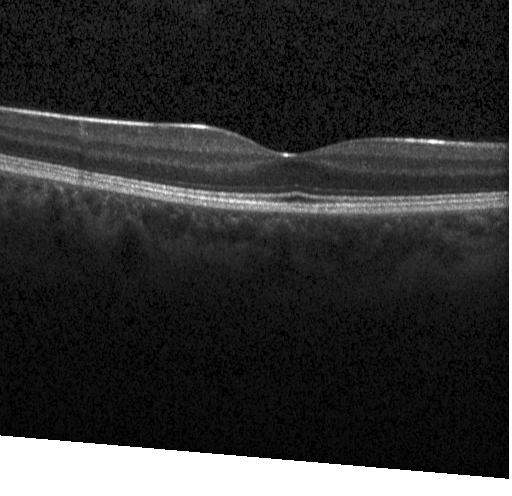

Finding: neither choroidal neovascularization, diabetic macular edema, nor drusen.